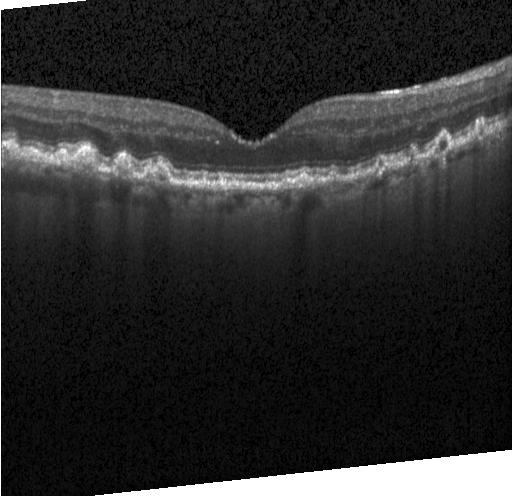 Acquired on a Heidelberg Spectralis. Spectral-domain OCT. OCT B-scan.
Impression: drusen.